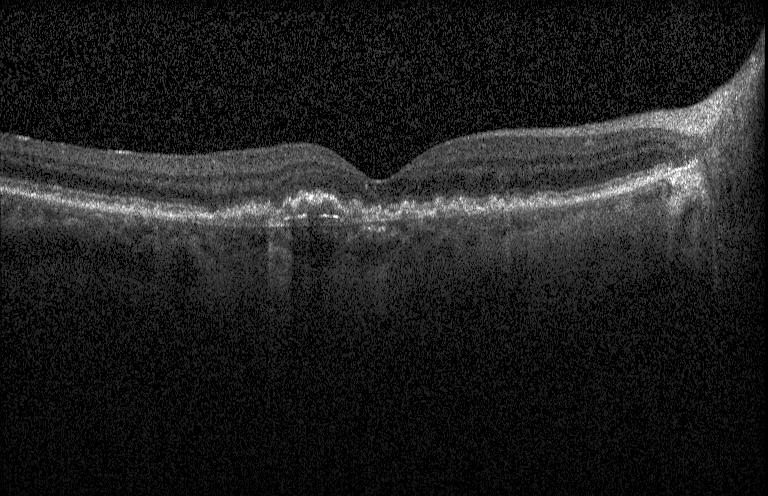
OCT B-scan showing choroidal neovascularization (CNV).